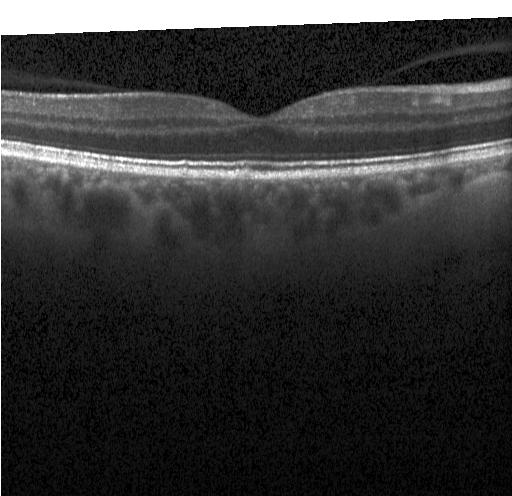 Centered on the fovea. OCT B-scan. Spectral-domain OCT.
OCT finding: neither choroidal neovascularization, diabetic macular edema, nor drusen.